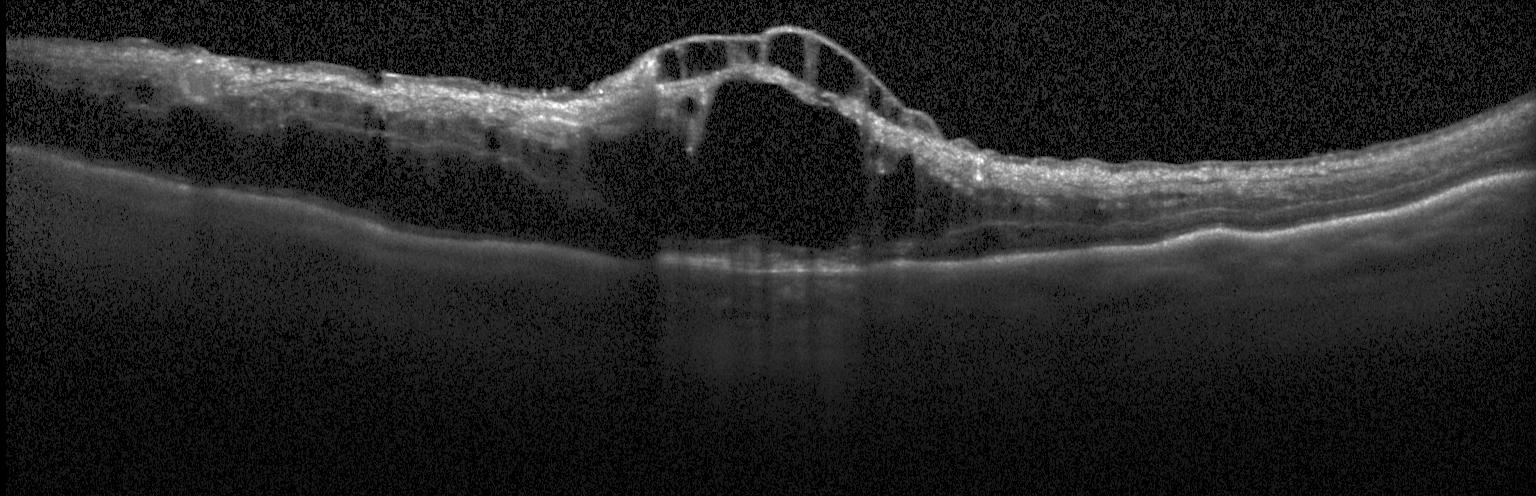

Finding: DME.